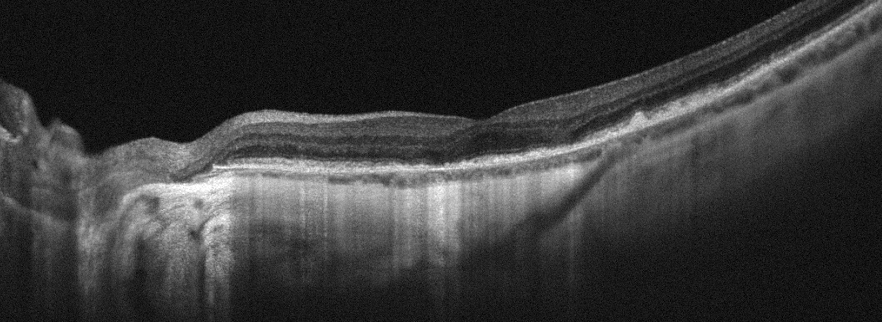
Optical coherence tomography scan, through the macula — Finding: age-related macular degeneration (AMD).